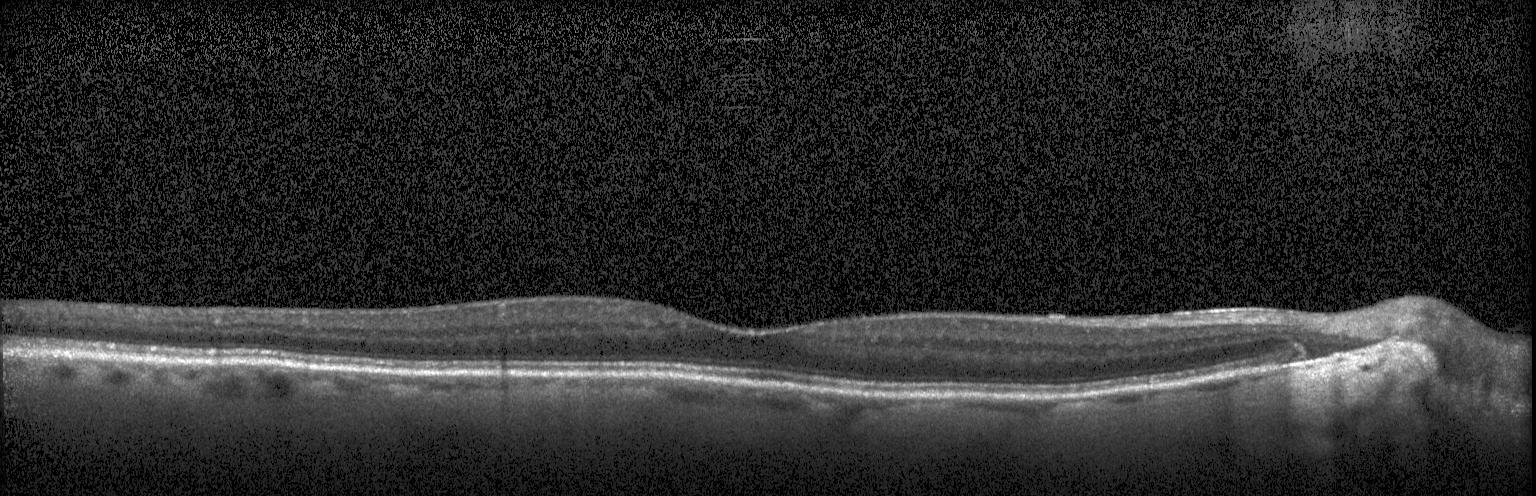 OCT line scan.
Diagnosis: neither choroidal neovascularization, diabetic macular edema, nor drusen.